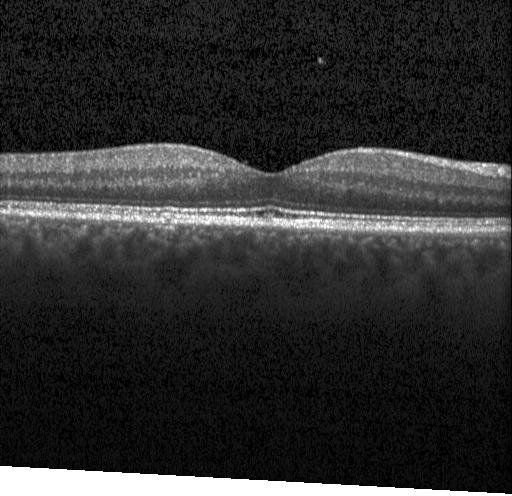 OCT B-scan
Diagnosis: neither choroidal neovascularization, diabetic macular edema, nor drusen.